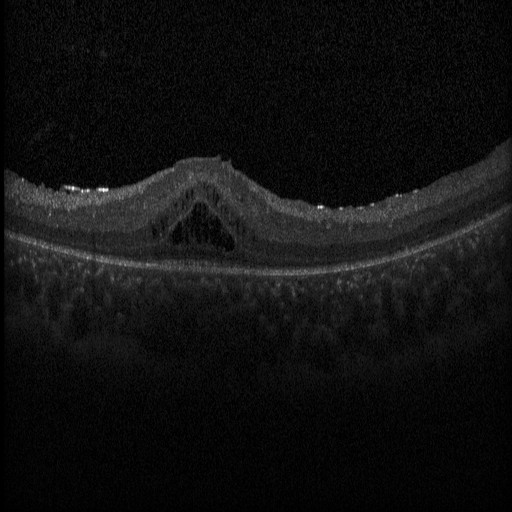
Retinal OCT cross-section. Macular scan. Acquired on a Heidelberg Spectralis. Spectral-domain OCT
Finding: diabetic macular edema.